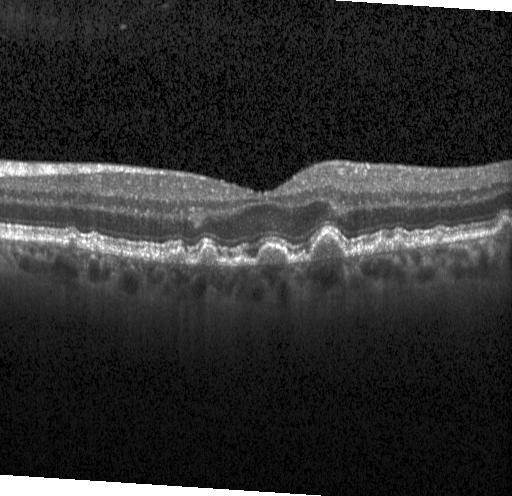 Retinal OCT cross-section showing drusen.